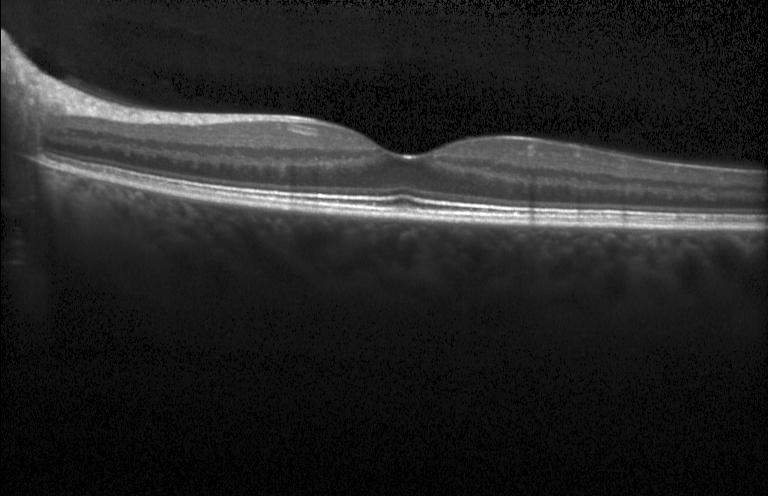

Optical coherence tomography B-scan; instrument: Heidelberg Spectralis; centered on the fovea; spectral-domain OCT.
Finding: no evidence of choroidal neovascularization, diabetic macular edema, or drusen.